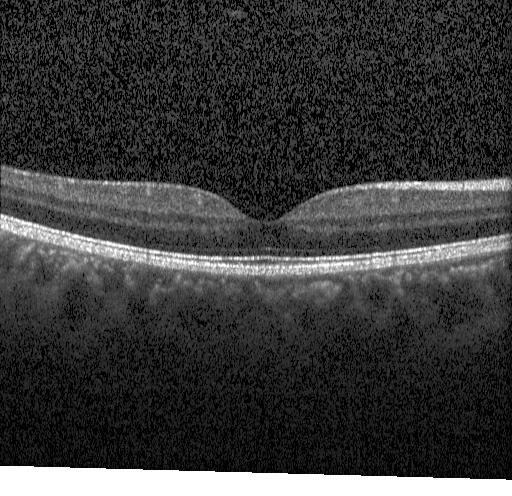

Finding: no choroidal neovascularization, diabetic macular edema, or drusen.